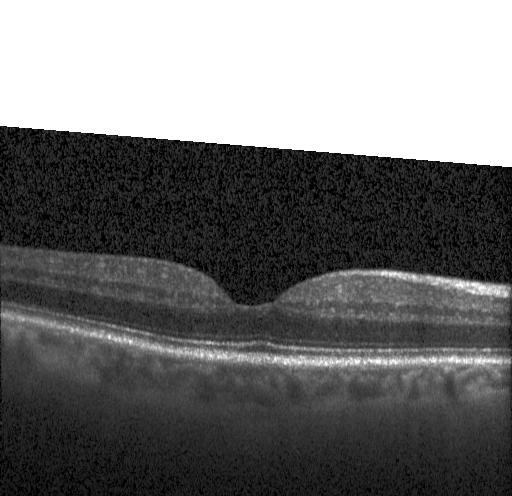 Optical coherence tomography scan.
The scan shows no evidence of choroidal neovascularization, diabetic macular edema, or drusen.